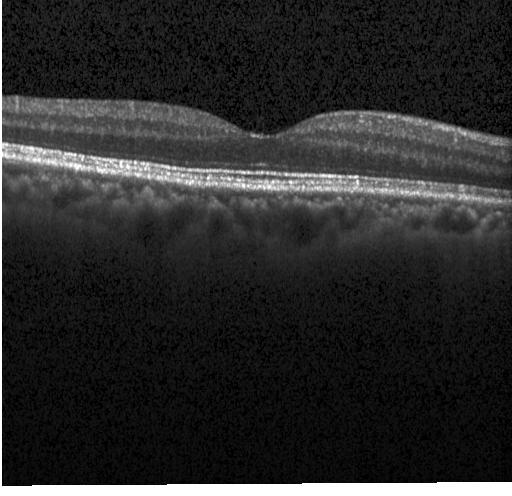
SD-OCT; Heidelberg Spectralis; retinal OCT B-scan. OCT finding: no choroidal neovascularization, no diabetic macular edema, and no drusen.